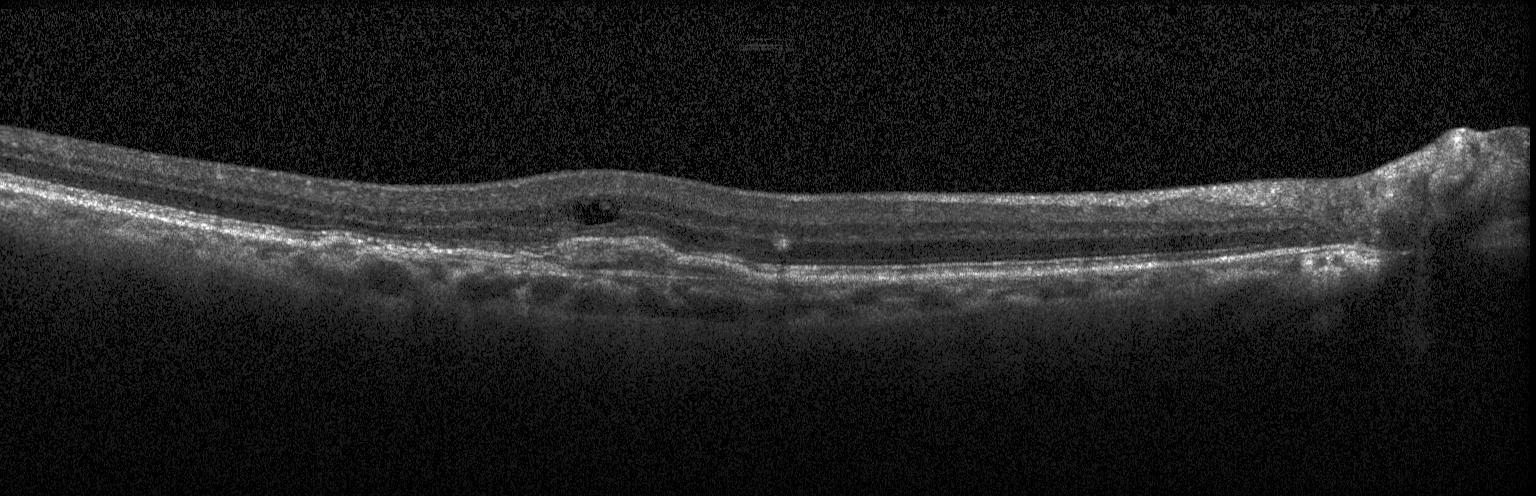
OCT line scan · acquired on a Heidelberg Spectralis · spectral-domain OCT.
The scan shows a choroidal neovascular membrane.